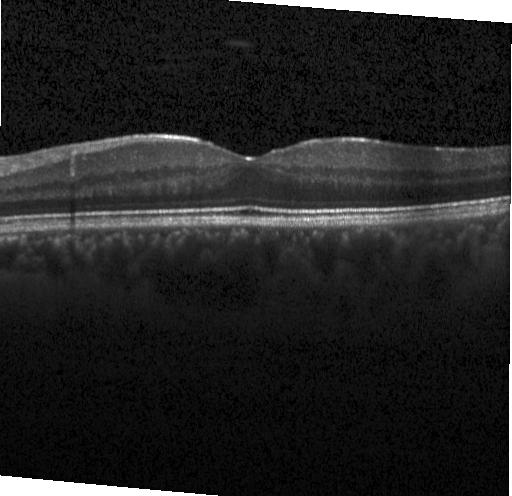
The scan shows neither choroidal neovascularization, diabetic macular edema, nor drusen.